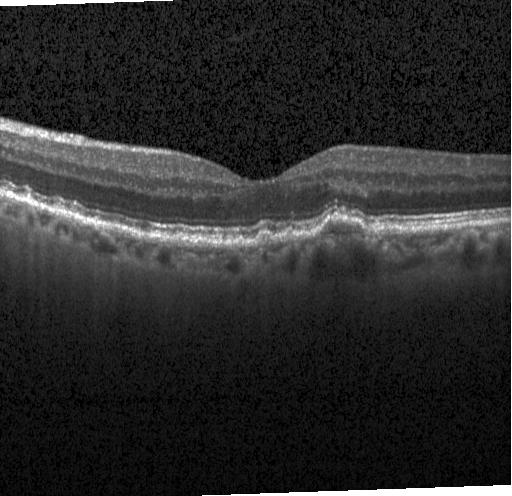 OCT B-scan
OCT finding: multiple drusen.